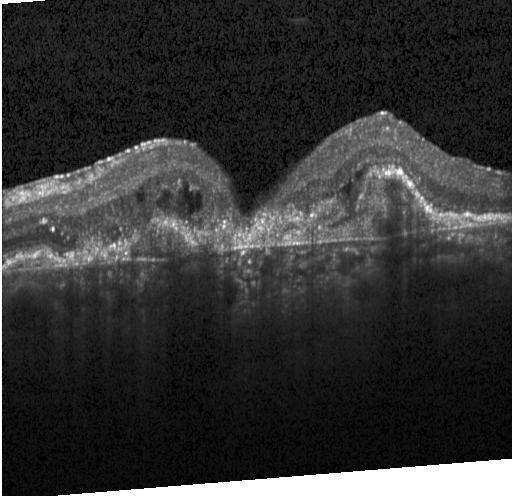
Horizontal scan through the fovea; spectral-domain optical coherence tomography; retinal OCT B-scan
The scan shows a choroidal neovascular membrane.